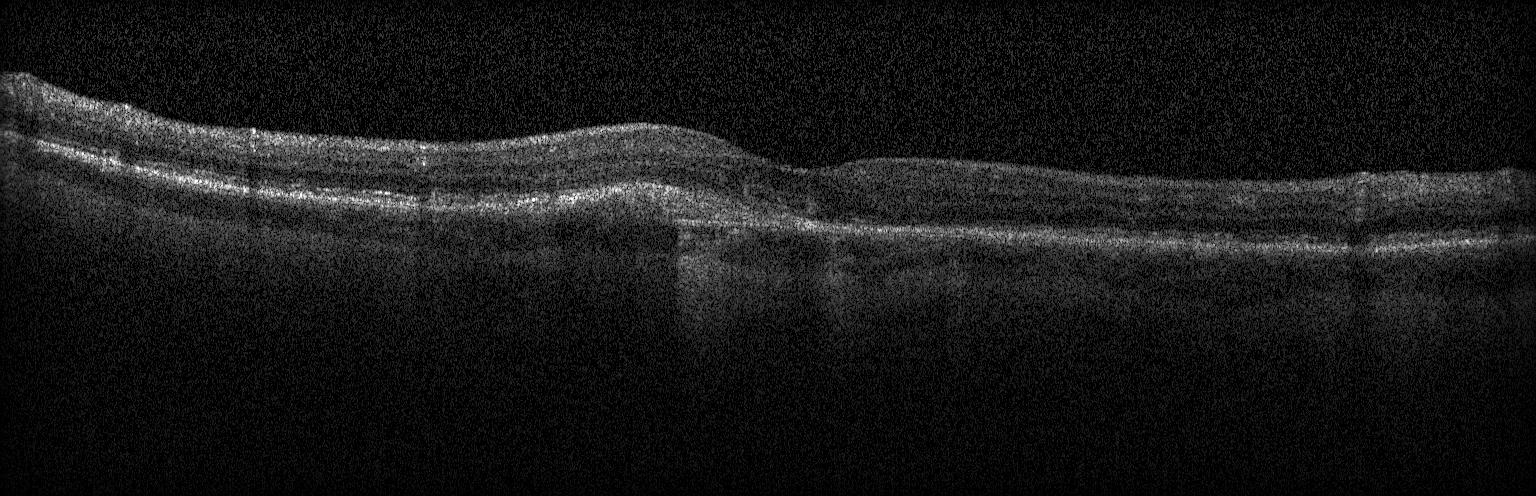

Acquired on a Heidelberg Spectralis; OCT line scan; spectral-domain OCT
This B-scan demonstrates a choroidal neovascular membrane.